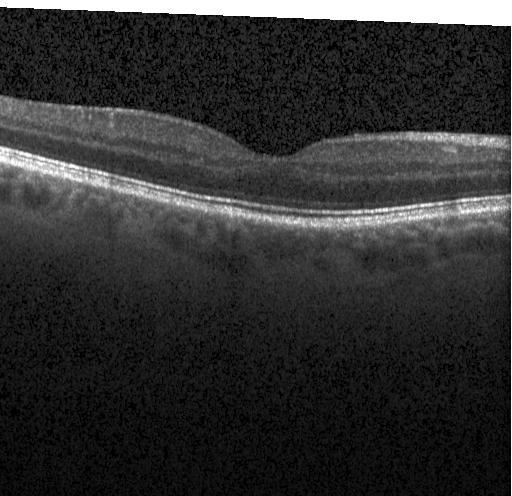 Impression: no choroidal neovascularization, no diabetic macular edema, and no drusen.